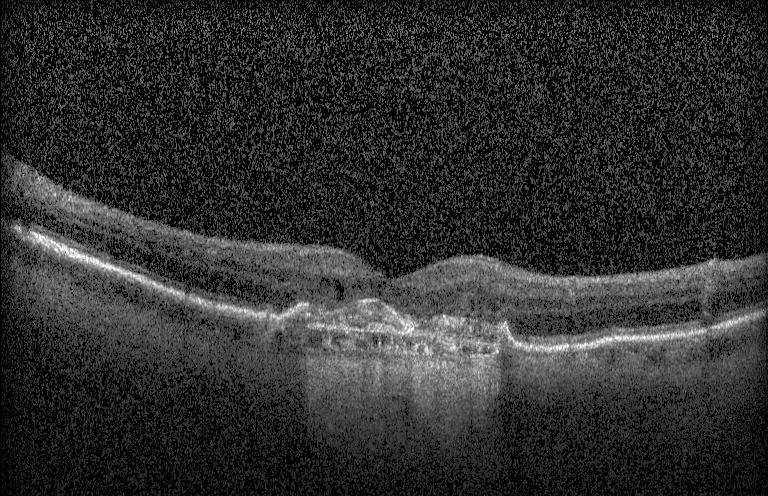 Heidelberg Spectralis OCT system, centered on the fovea, retinal OCT cross-section, spectral-domain optical coherence tomography — Macular OCT: choroidal neovascularization (CNV).